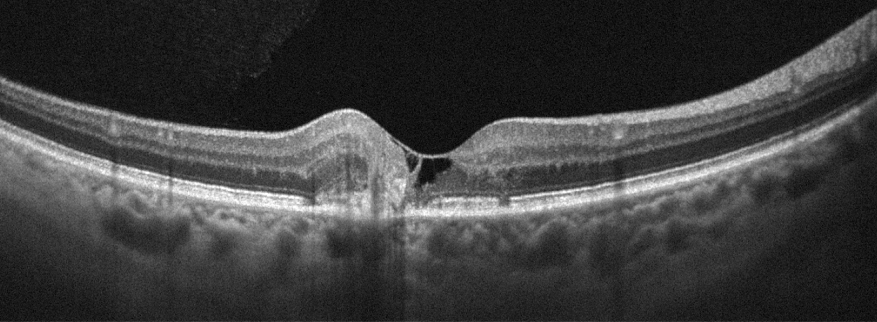

Optical coherence tomography B-scan — Diagnosis: age-related macular degeneration.